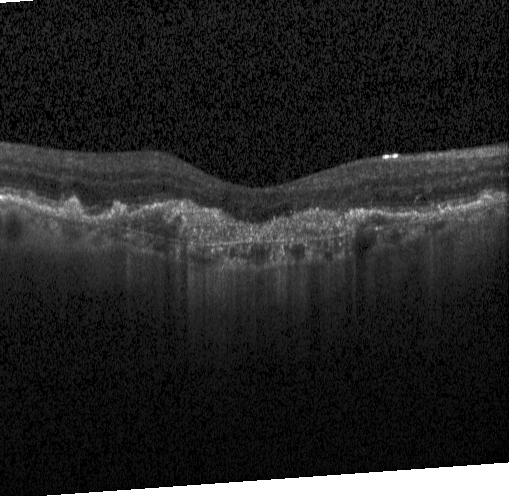

Spectral-domain OCT · OCT line scan. Diagnosis: a choroidal neovascular membrane.